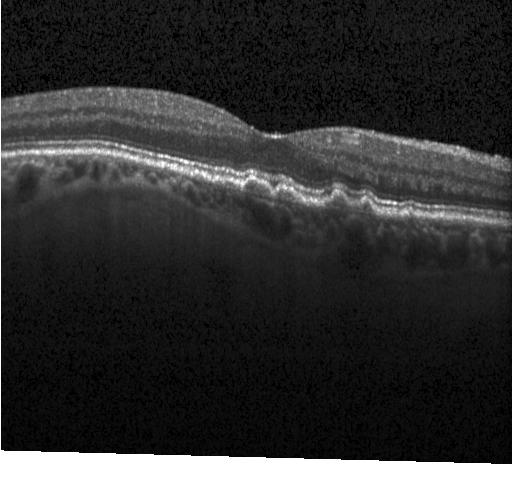

Spectral-domain optical coherence tomography, acquired on a Heidelberg Spectralis, retinal OCT cross-section — OCT finding: sub-RPE drusenoid deposits.